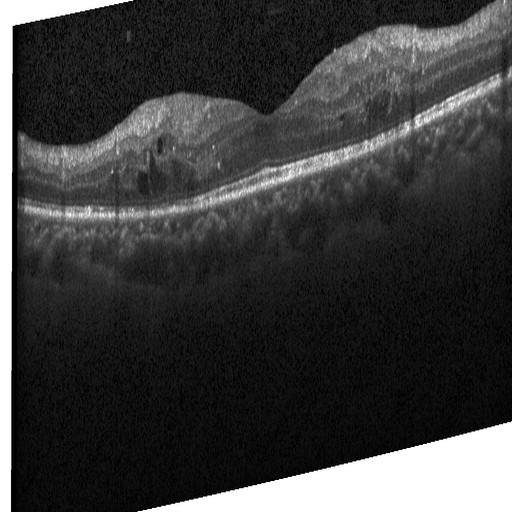
Finding: DME.